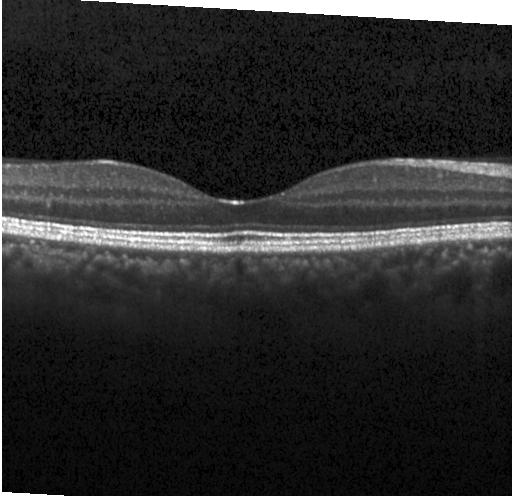 Instrument: Heidelberg Spectralis · spectral-domain optical coherence tomography · macular scan · retinal OCT B-scan
This B-scan demonstrates neither choroidal neovascularization, diabetic macular edema, nor drusen.